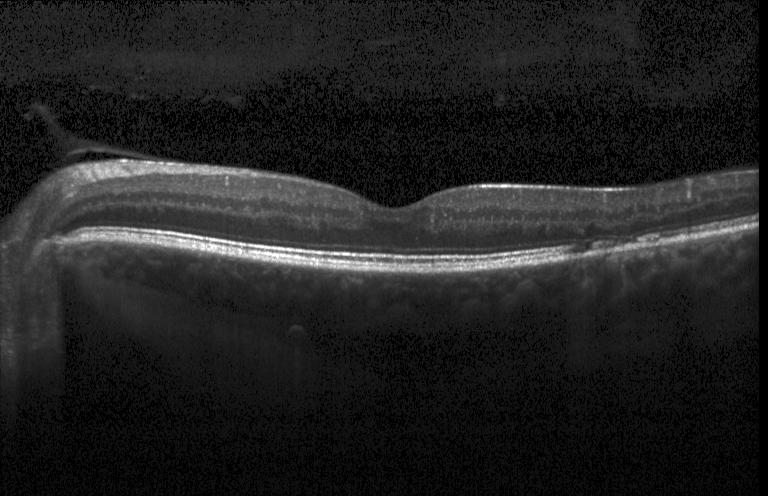 OCT line scan. Spectral-domain OCT.
Neither choroidal neovascularization, diabetic macular edema, nor drusen.